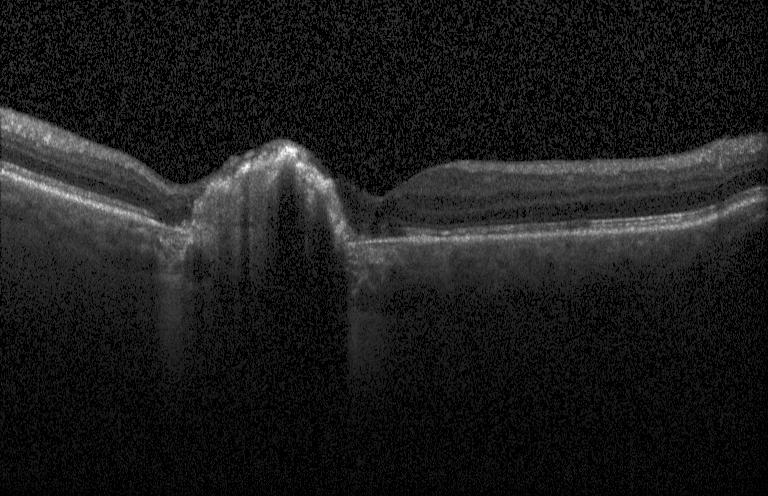

OCT scan showing a choroidal neovascular membrane.